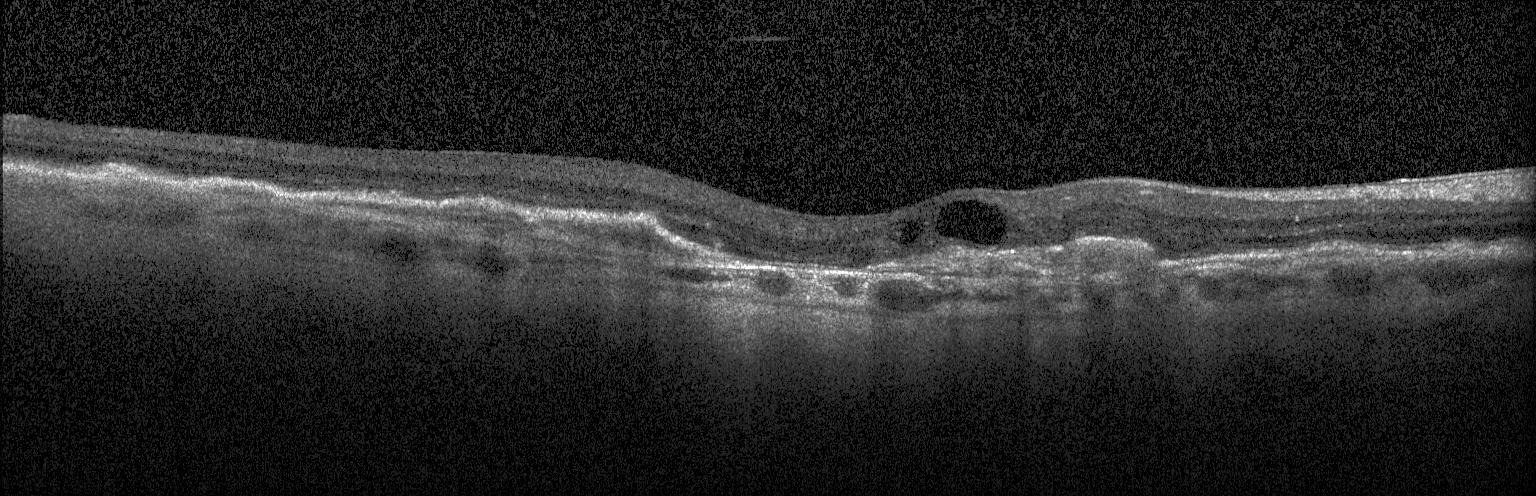

OCT B-scan. Heidelberg Spectralis. Spectral-domain optical coherence tomography.
Dx: choroidal neovascularization (CNV).